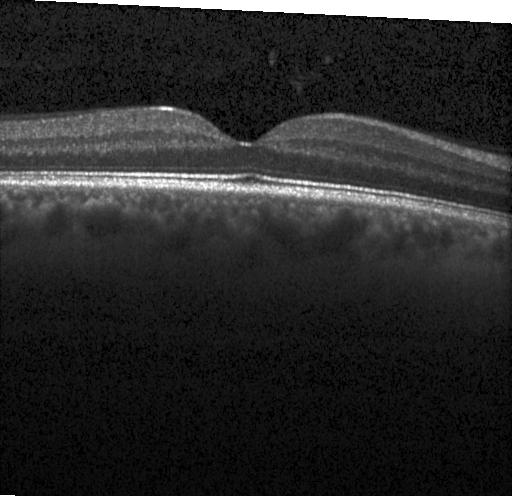

Retinal OCT B-scan — Impression: no choroidal neovascularization, diabetic macular edema, or drusen.